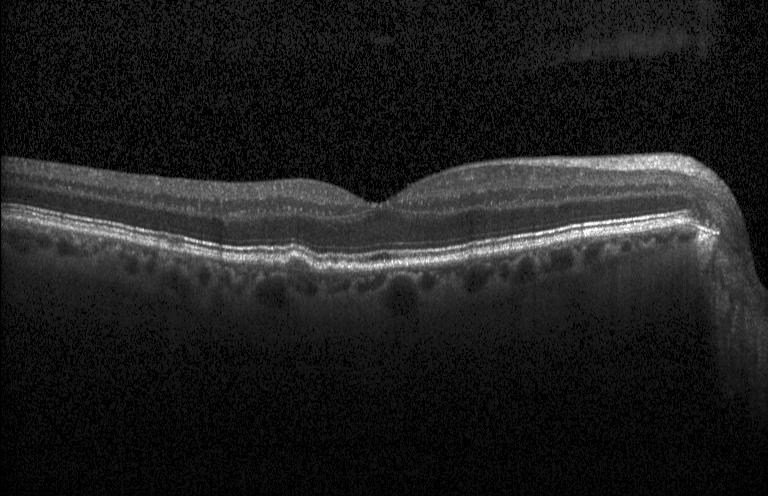

Horizontal scan through the fovea, OCT line scan, spectral-domain OCT. Assessment: drusen.